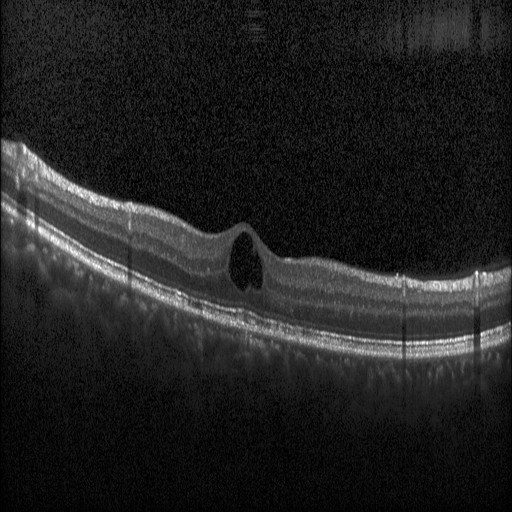

Finding: diabetic macular edema.